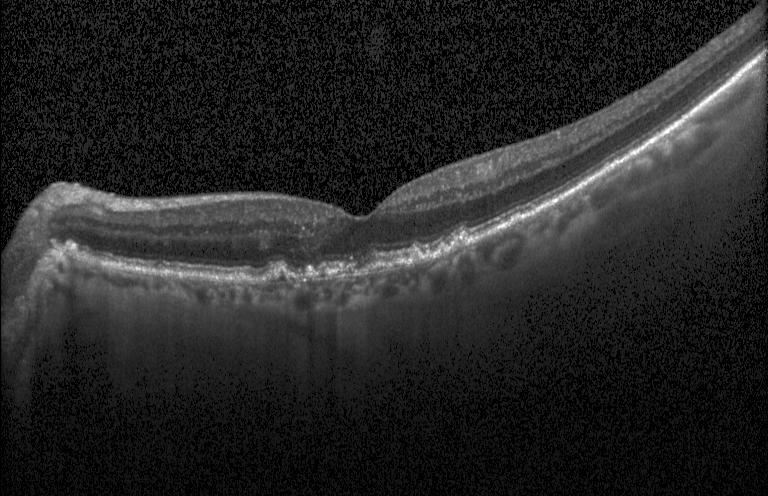 OCT line scan, fovea-centered — Impression: sub-RPE drusenoid deposits.